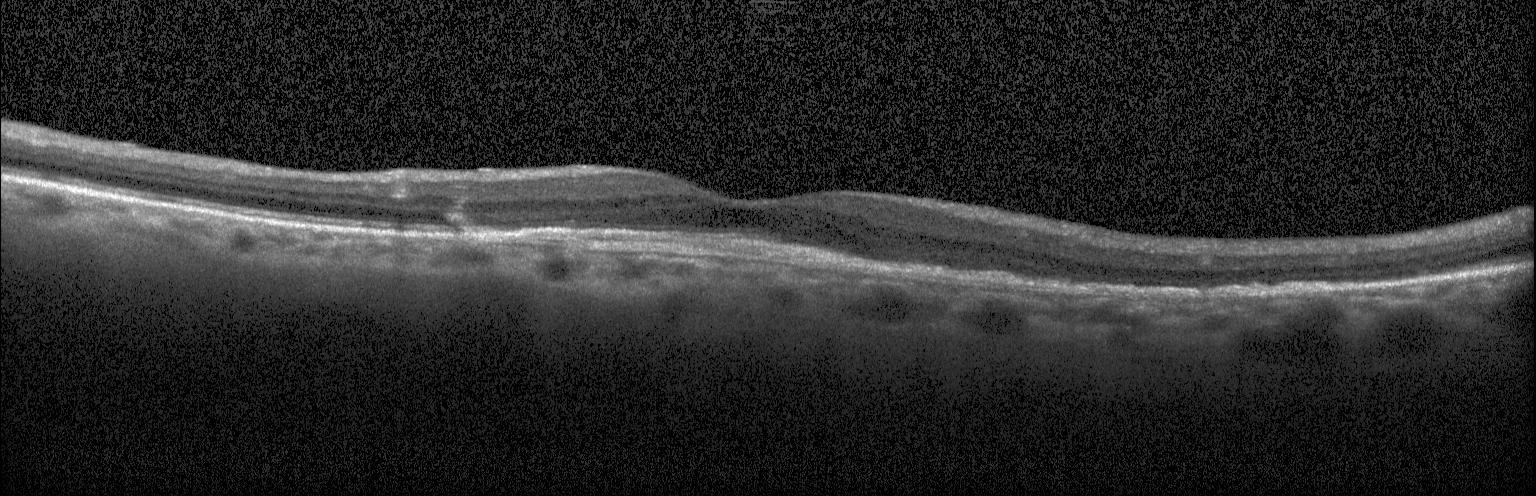

Optical coherence tomography scan
Finding: a choroidal neovascular membrane.